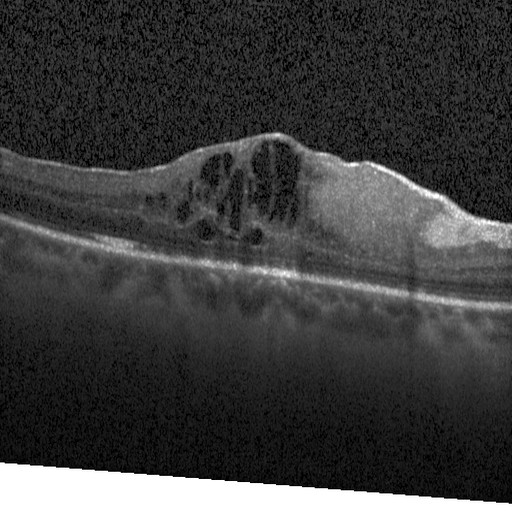

Optical coherence tomography scan.
This B-scan demonstrates DME.